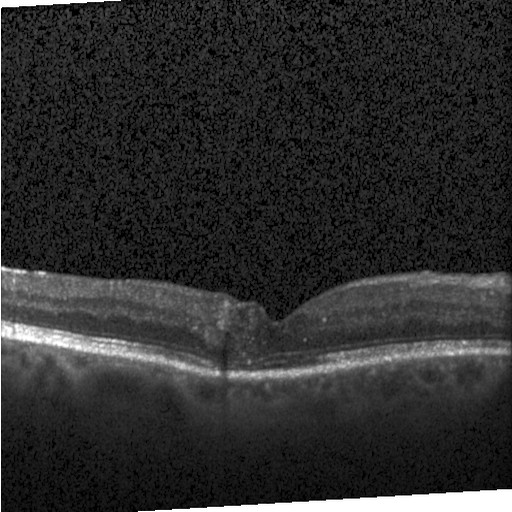

Spectral-domain optical coherence tomography · retinal OCT cross-section · macular scan.
The scan shows diabetic macular edema (DME).